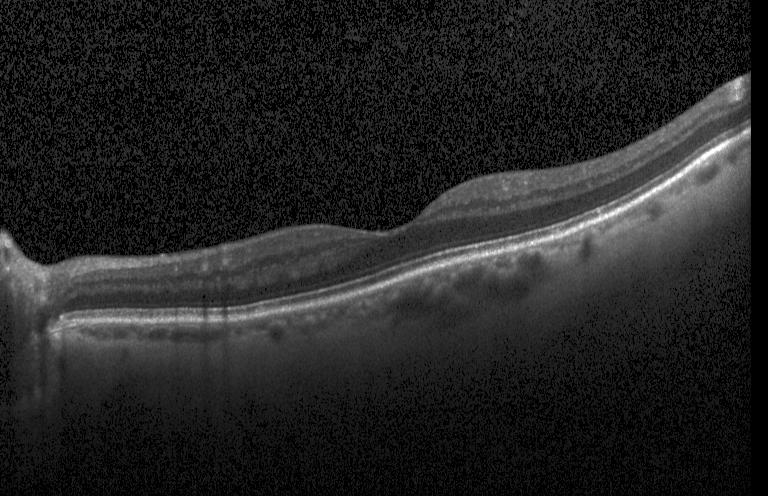

OCT finding: no evidence of CNV, DME, or drusen.